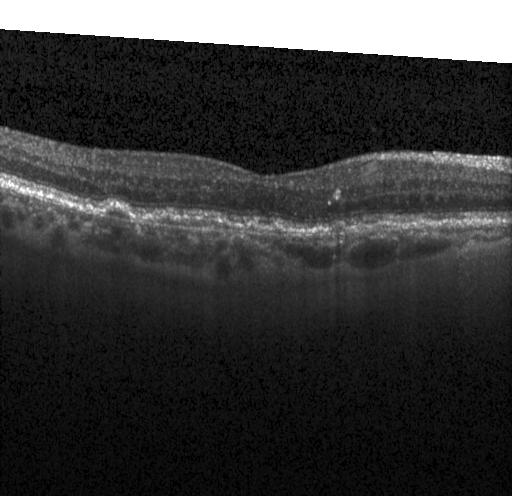
Retinal OCT B-scan
Impression: CNV.